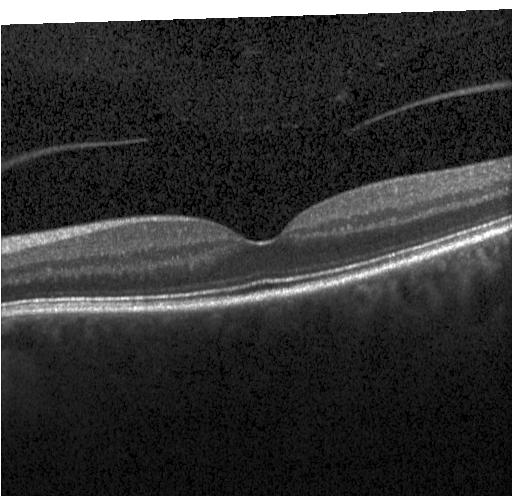

Finding: neither CNV, DME, nor drusen.